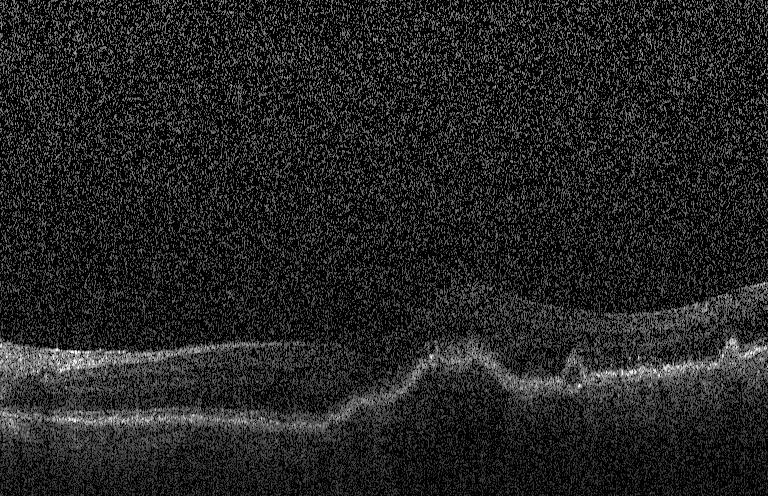
Retinal OCT cross-section showing choroidal neovascularization.